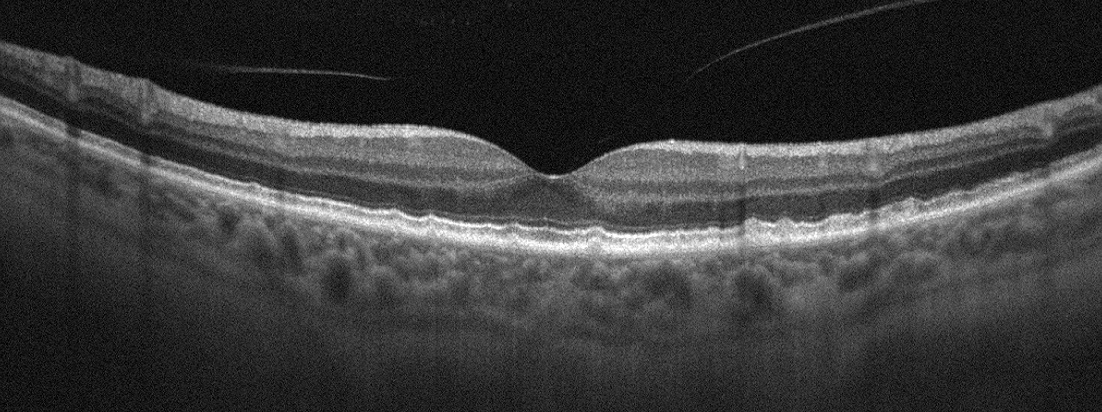
This B-scan demonstrates AMD.